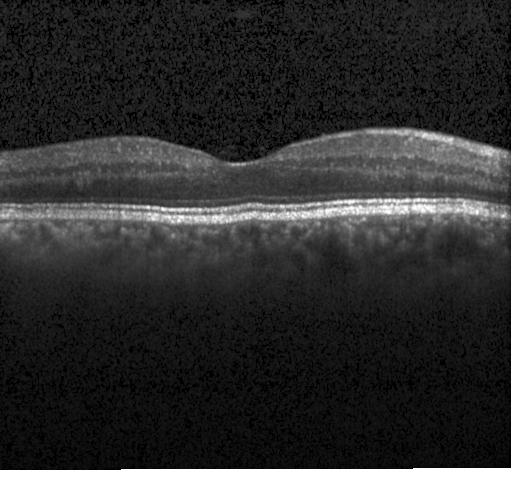 Optical coherence tomography scan — The scan shows no choroidal neovascularization, no diabetic macular edema, and no drusen.